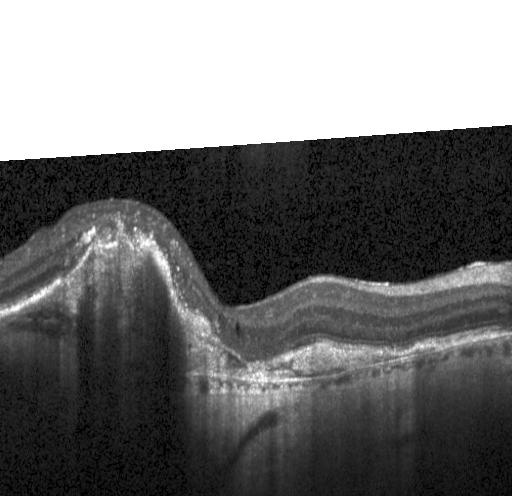 SD-OCT; OCT line scan — The scan shows a choroidal neovascular membrane.